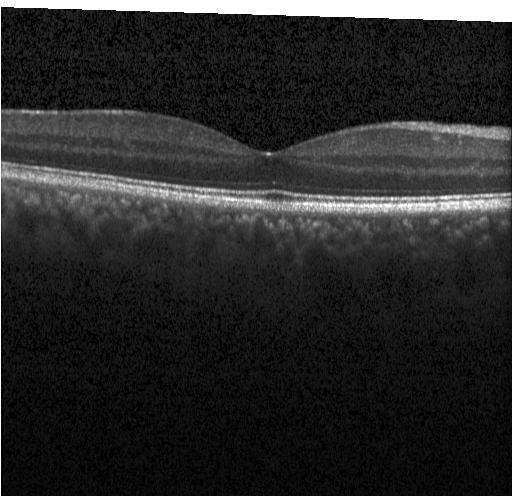
Dx: no choroidal neovascularization, diabetic macular edema, or drusen.